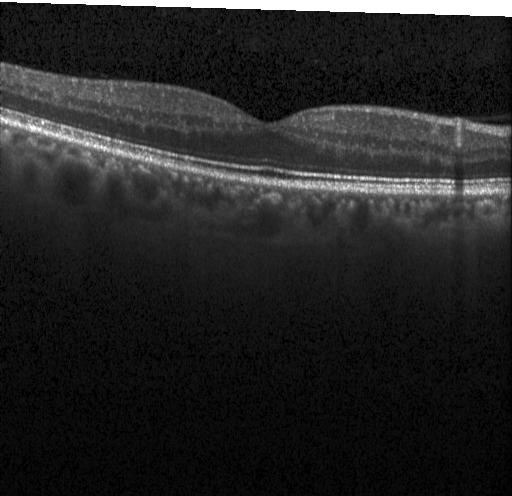

Optical coherence tomography B-scan
Finding: no choroidal neovascularization, no diabetic macular edema, and no drusen.